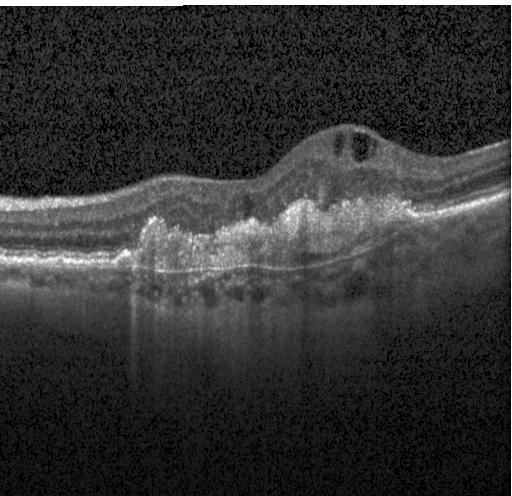 OCT B-scan · Heidelberg Spectralis OCT system.
Dx: a choroidal neovascular membrane.